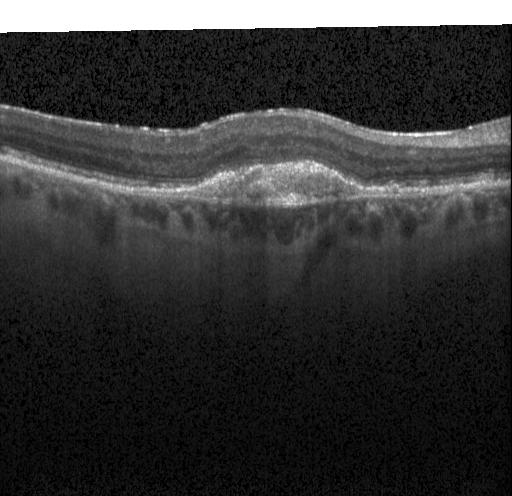 OCT finding: a choroidal neovascular membrane.